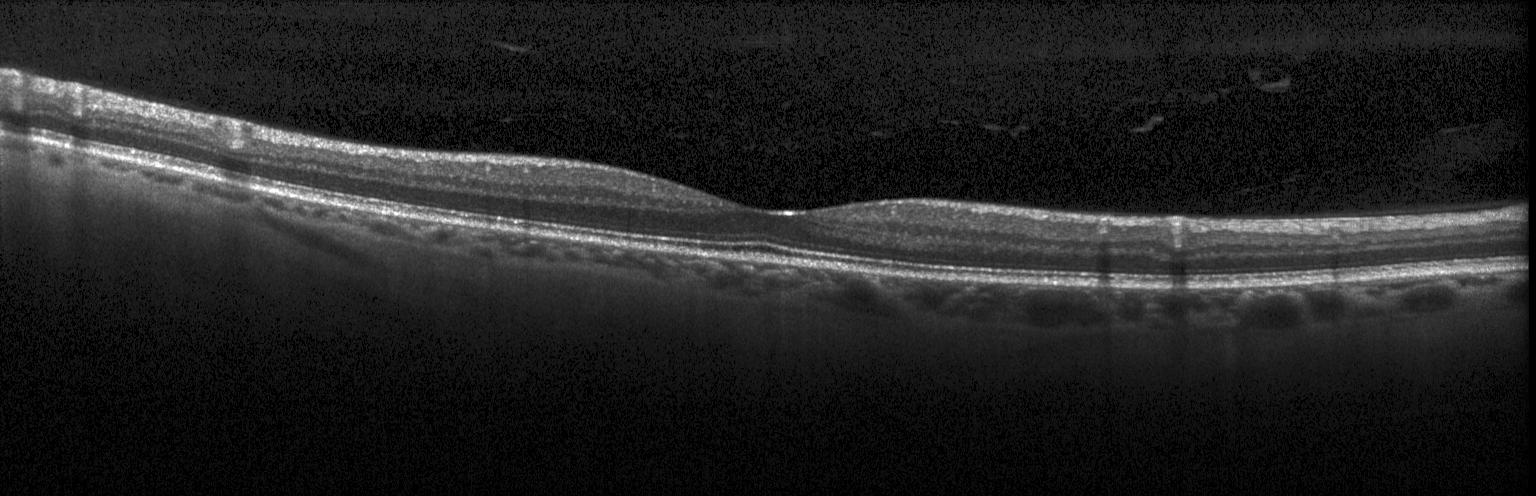
Macular OCT: no evidence of CNV, DME, or drusen.